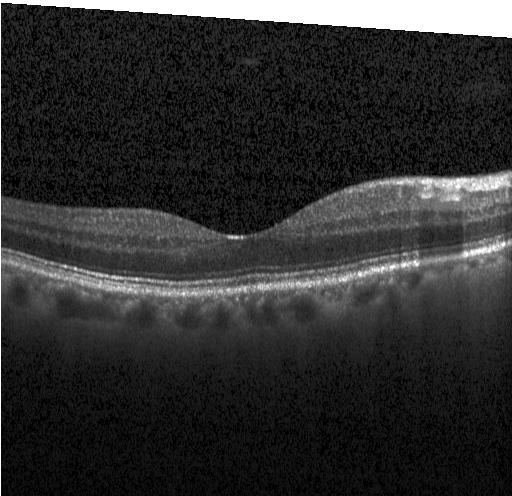

Fovea-centered. Heidelberg Spectralis. Retinal OCT cross-section. SD-OCT.
Impression: neither choroidal neovascularization, diabetic macular edema, nor drusen.